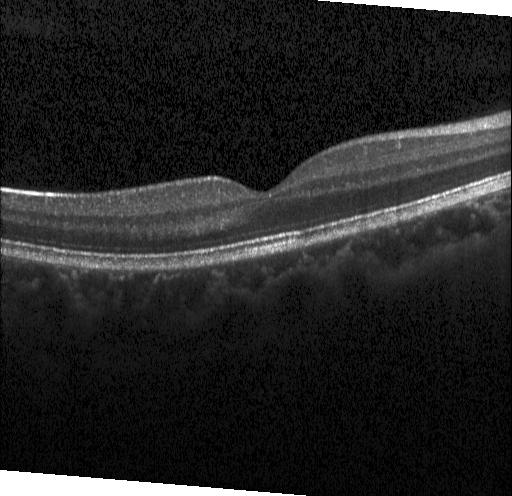
This B-scan demonstrates neither CNV, DME, nor drusen.